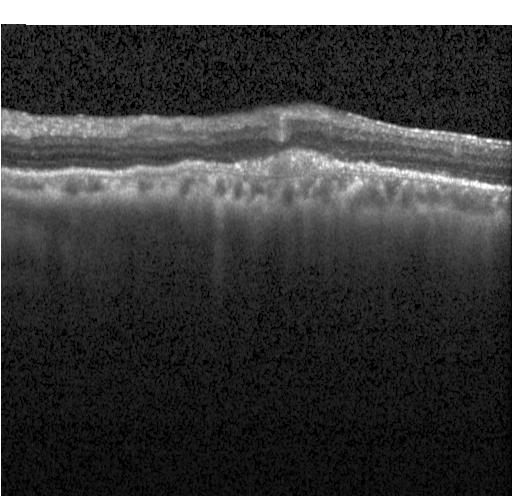

Impression: a choroidal neovascular membrane.